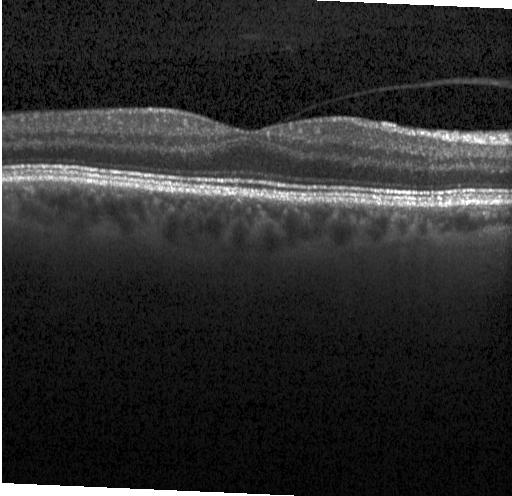 OCT B-scan showing no evidence of choroidal neovascularization, diabetic macular edema, or drusen.